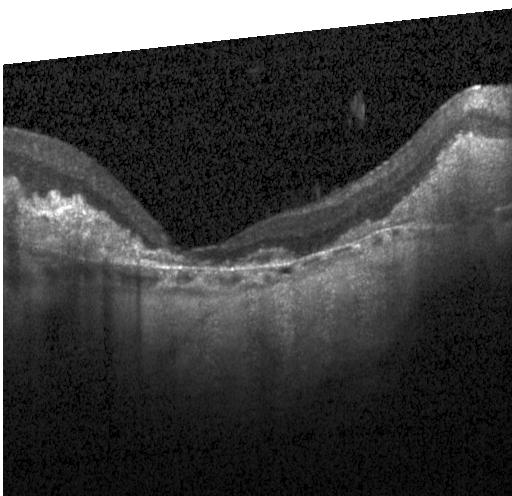 Optical coherence tomography B-scan.
Impression: CNV.